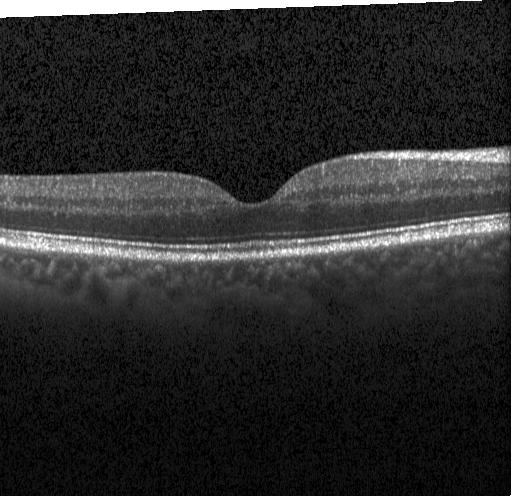

Optical coherence tomography B-scan, fovea-centered, acquired on a Heidelberg Spectralis, SD-OCT. Finding: no evidence of choroidal neovascularization, diabetic macular edema, or drusen.